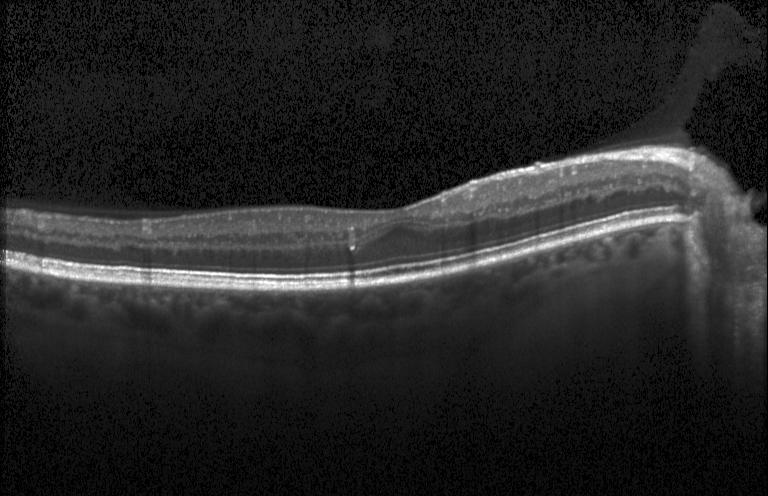
Retinal OCT B-scan · spectral-domain OCT — The scan shows no choroidal neovascularization, no diabetic macular edema, and no drusen.